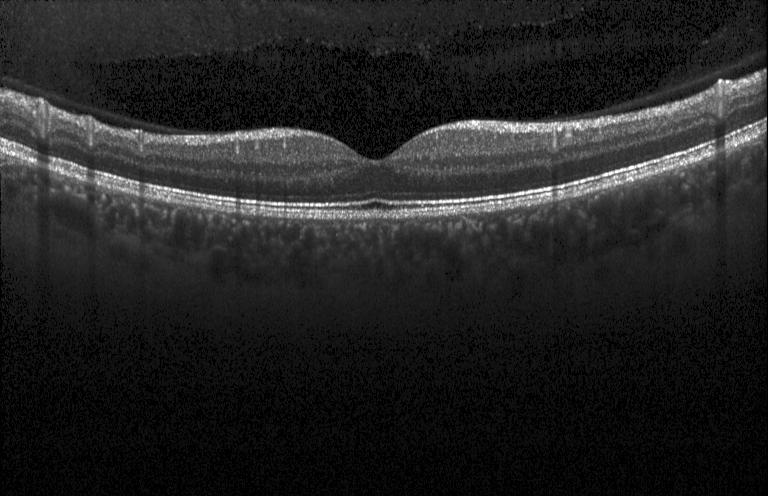

Macular OCT: neither CNV, DME, nor drusen.